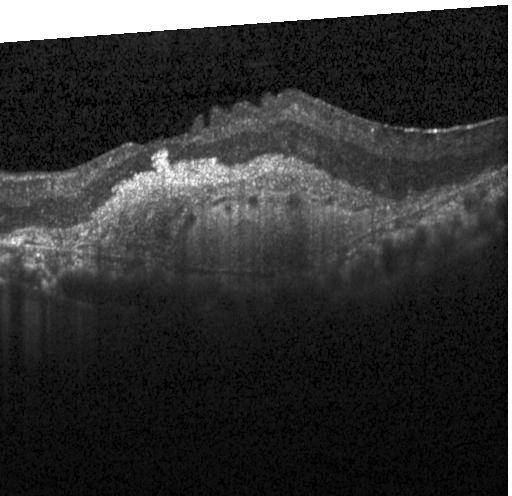 Retinal OCT cross-section. Spectral-domain OCT. Impression: choroidal neovascularization.